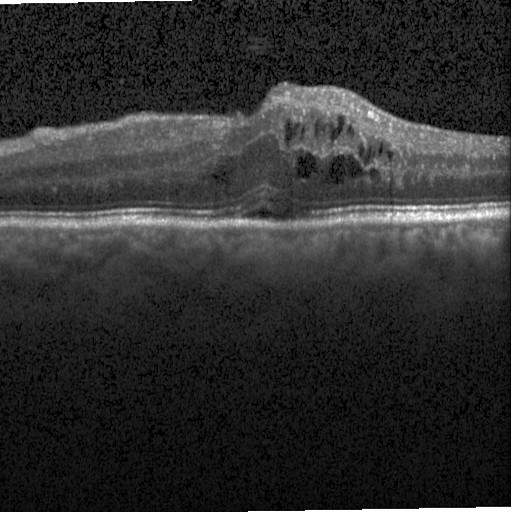

OCT B-scan. Heidelberg Spectralis. Diabetic macular edema.